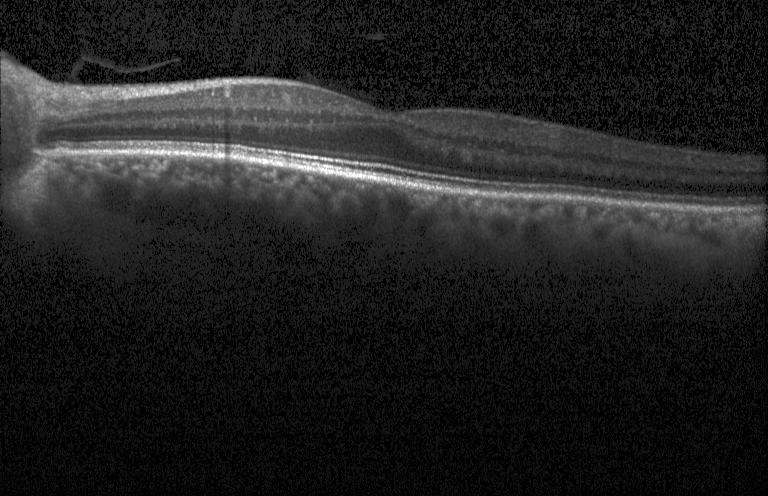 OCT B-scan, fovea-centered
Impression: no evidence of choroidal neovascularization, diabetic macular edema, or drusen.